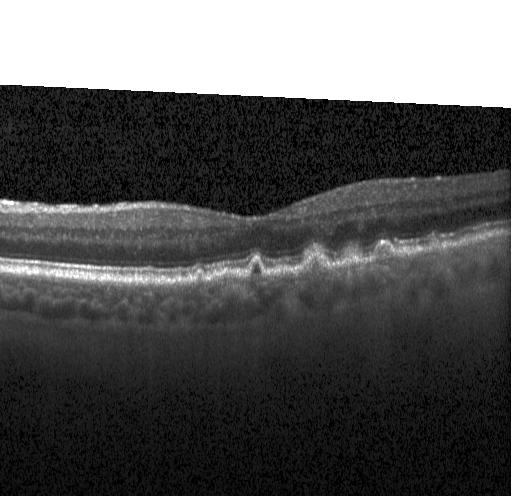

Spectral-domain OCT · horizontal scan through the fovea · retinal OCT cross-section · acquired on a Heidelberg Spectralis.
Finding: drusen.